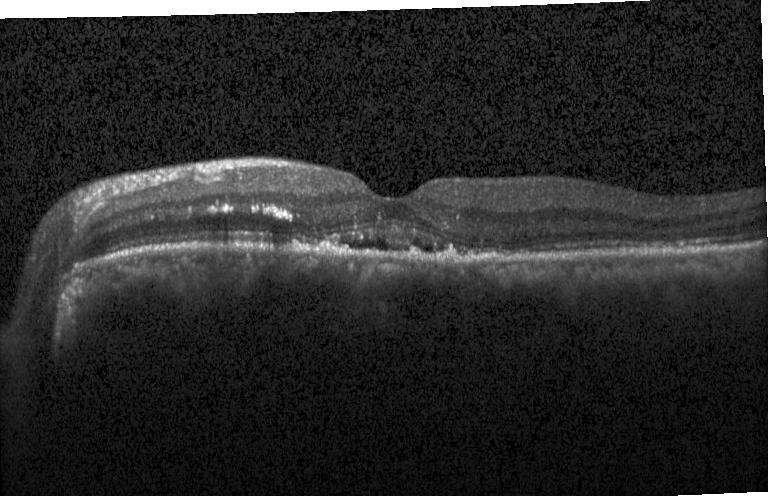

Retinal OCT B-scan; SD-OCT. The scan shows choroidal neovascularization.